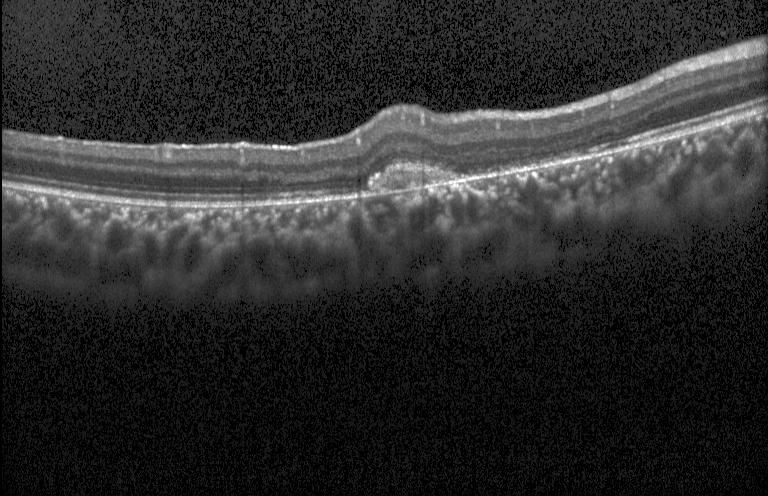
CNV.